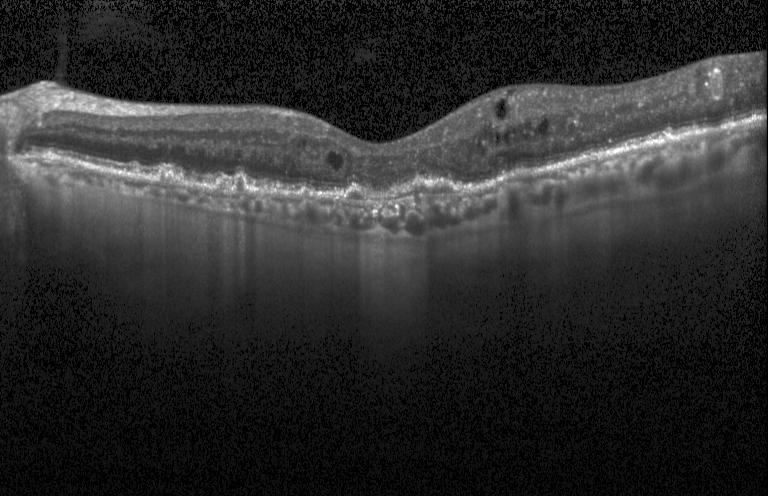 Retinal OCT B-scan.
Assessment: a choroidal neovascular membrane.